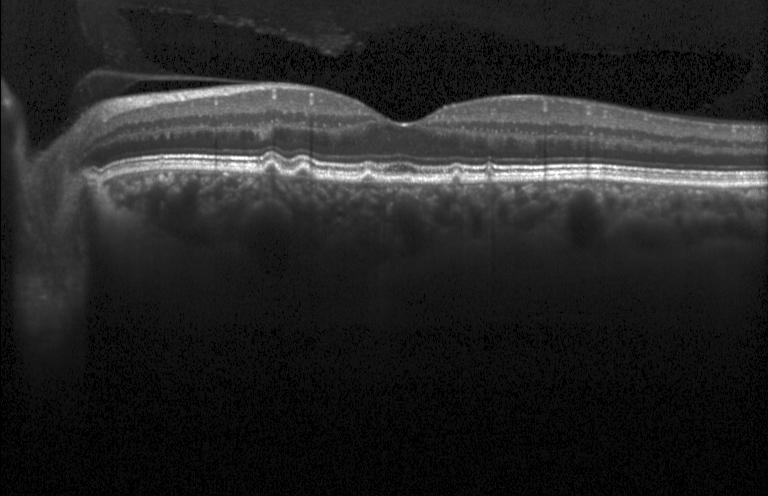 Optical coherence tomography B-scan; Heidelberg Spectralis
Drusen.